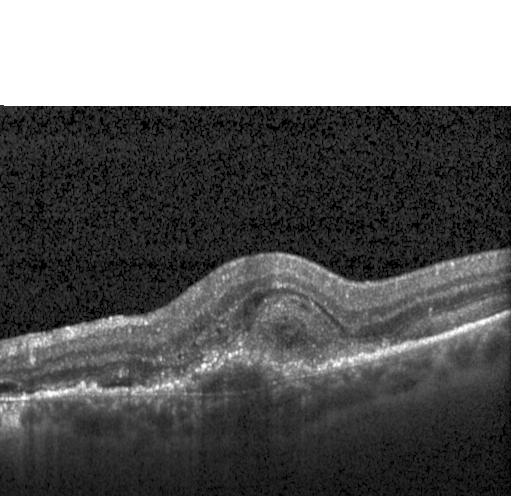
Retinal OCT cross-section showing CNV.